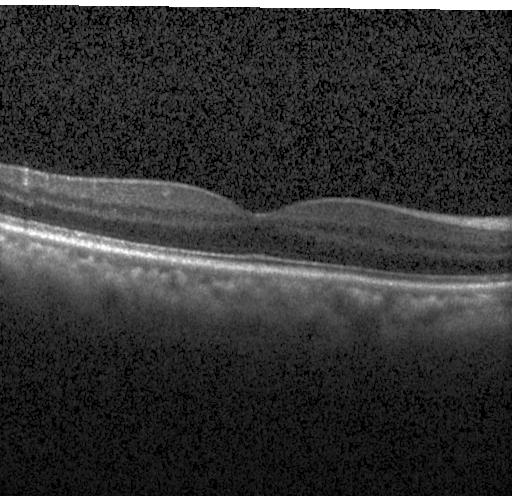

Acquired on a Heidelberg Spectralis. Retinal OCT B-scan
Assessment: neither CNV, DME, nor drusen.